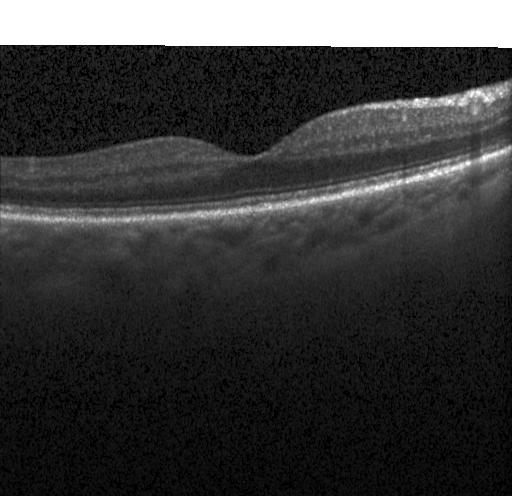

Diagnosis: no CNV, DME, or drusen.